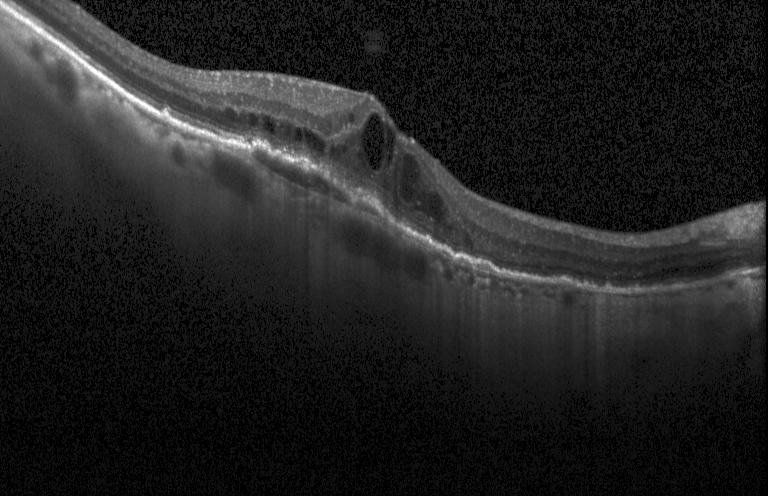 Fovea-centered, retinal OCT cross-section — Assessment: a choroidal neovascular membrane.